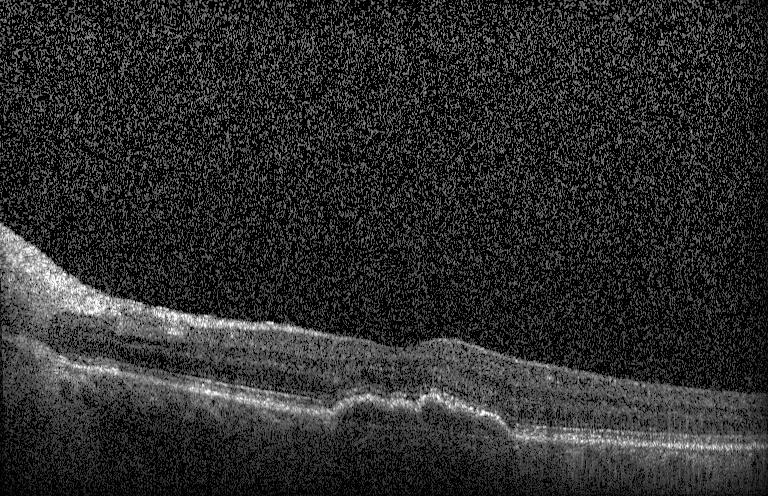
Centered on the fovea. SD-OCT. Heidelberg Spectralis OCT system. OCT B-scan.
Finding: a choroidal neovascular membrane.